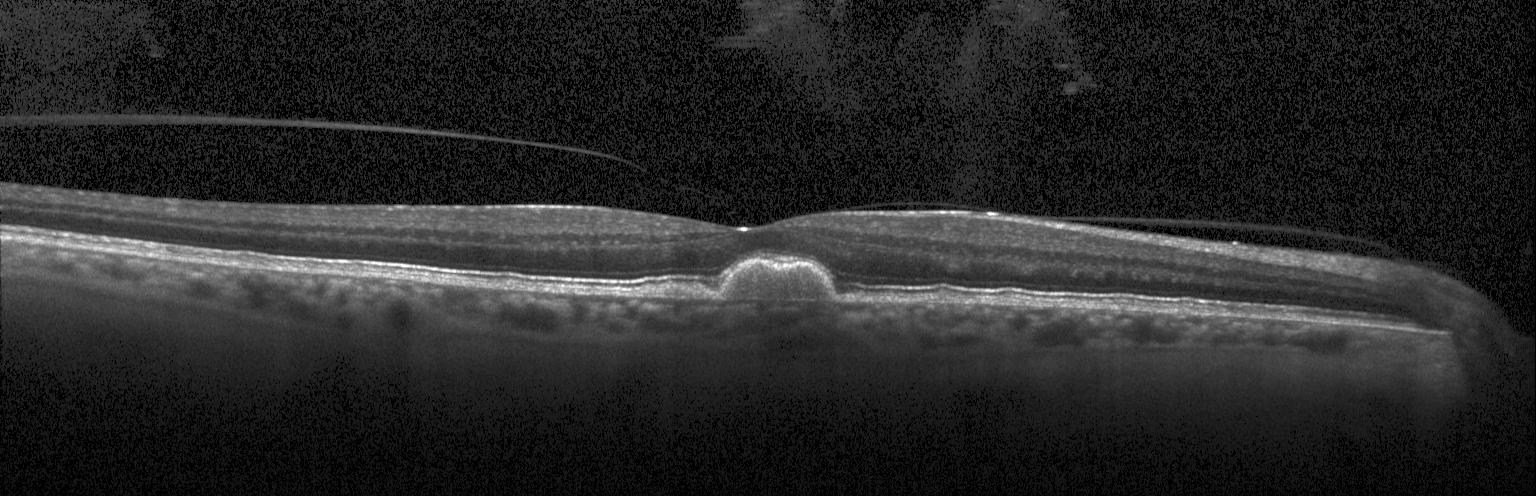 This B-scan demonstrates CNV.